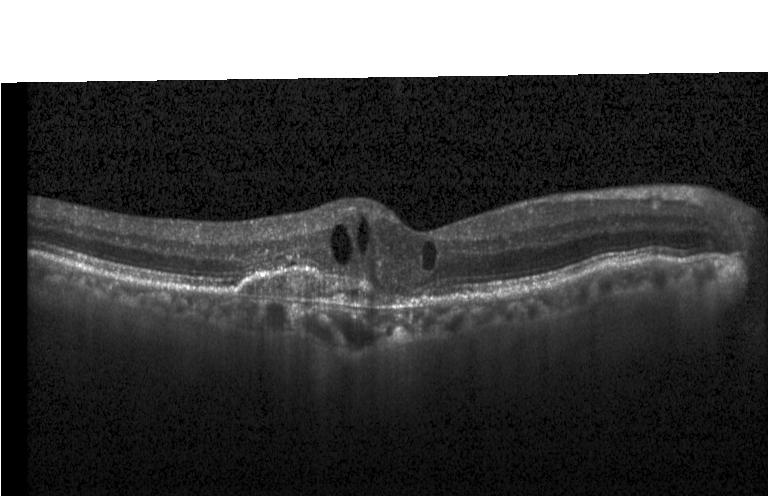 Spectral-domain optical coherence tomography, optical coherence tomography B-scan, instrument: Heidelberg Spectralis, horizontal scan through the fovea.
Impression: CNV.